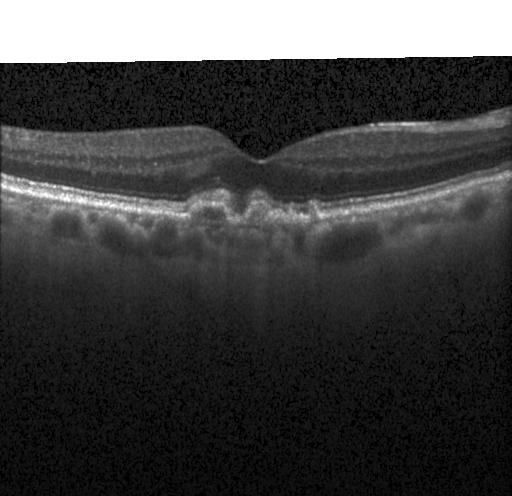

OCT line scan · instrument: Heidelberg Spectralis · SD-OCT · centered on the fovea
Diagnosis: choroidal neovascularization.